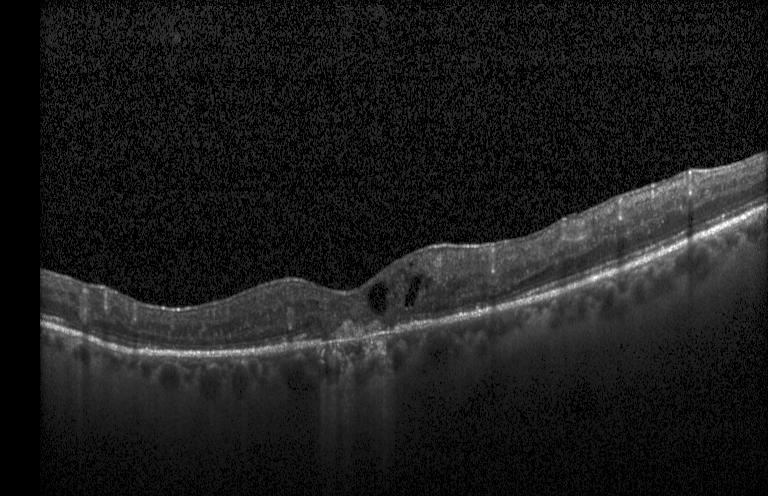

Finding: a choroidal neovascular membrane.